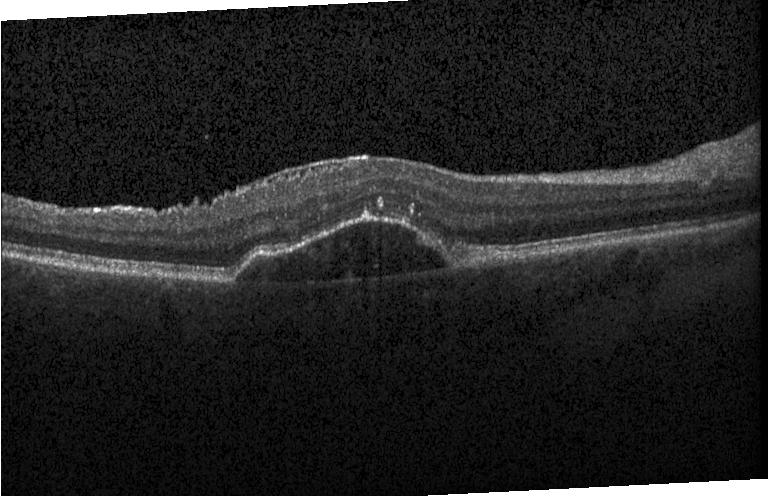

Fovea-centered. Acquired on a Heidelberg Spectralis. Retinal OCT B-scan.
Impression: choroidal neovascularization.